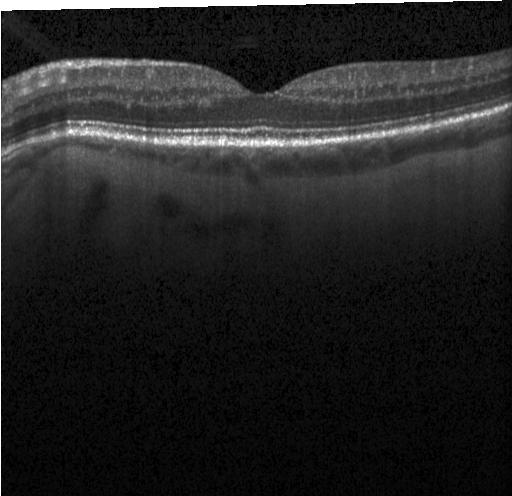
SD-OCT; optical coherence tomography scan.
Diagnosis: no CNV, DME, or drusen.